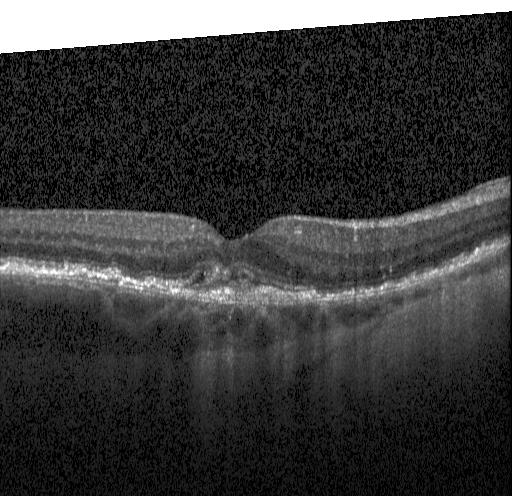 Acquired on a Heidelberg Spectralis; macular scan; optical coherence tomography B-scan; spectral-domain optical coherence tomography — Diagnosis: choroidal neovascularization (CNV).